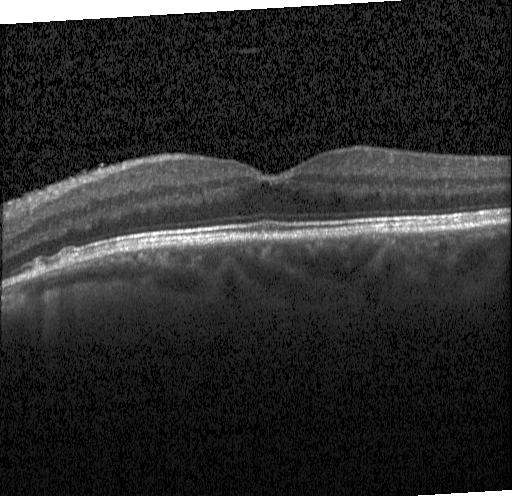 Heidelberg Spectralis; through the macula; retinal OCT cross-section. The scan shows no CNV, no DME, and no drusen.